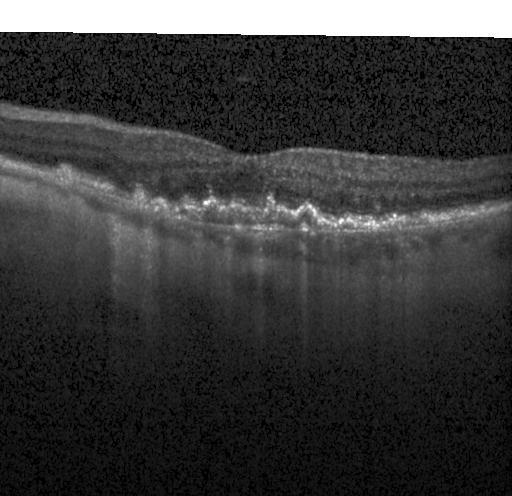
The scan shows a choroidal neovascular membrane.